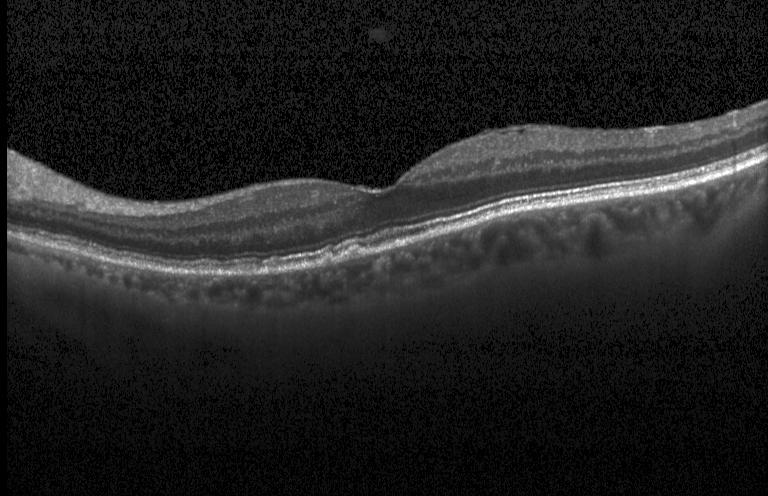

Optical coherence tomography scan, instrument: Heidelberg Spectralis, spectral-domain OCT
Assessment: multiple drusen.